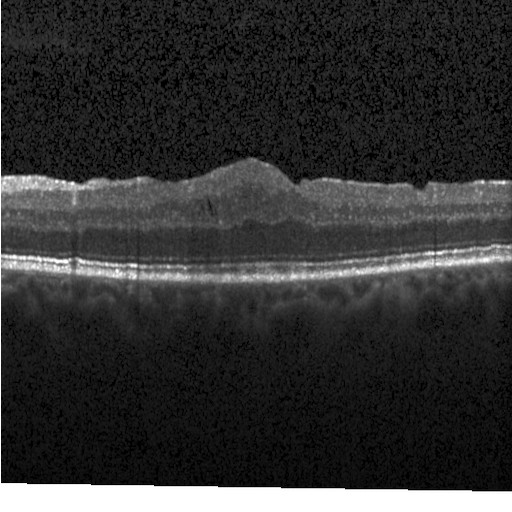
Macular OCT: diabetic macular edema (DME).